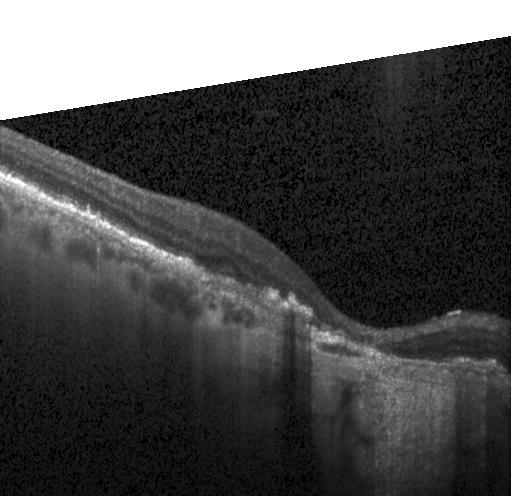

OCT B-scan. Assessment: a choroidal neovascular membrane.